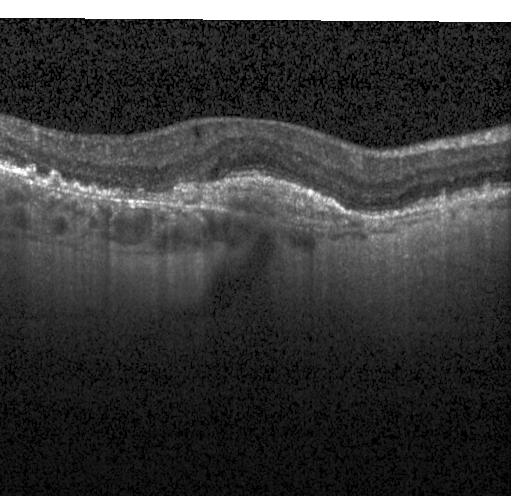

OCT B-scan · spectral-domain OCT · centered on the fovea · Heidelberg Spectralis OCT system. This B-scan demonstrates CNV.